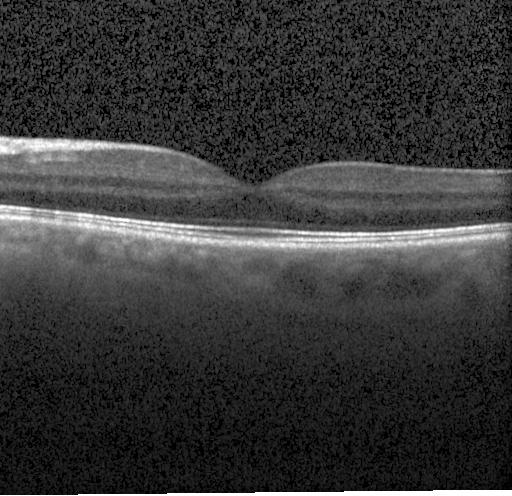 Heidelberg Spectralis OCT system · SD-OCT · OCT line scan
Impression: no choroidal neovascularization, no diabetic macular edema, and no drusen.